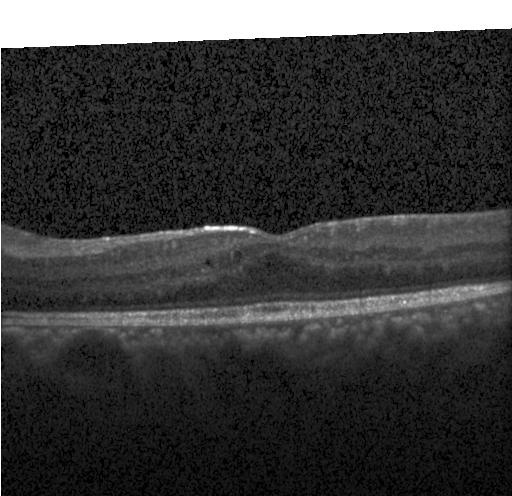
Spectral-domain OCT, optical coherence tomography scan, centered on the fovea.
Diagnosis: diabetic macular edema.